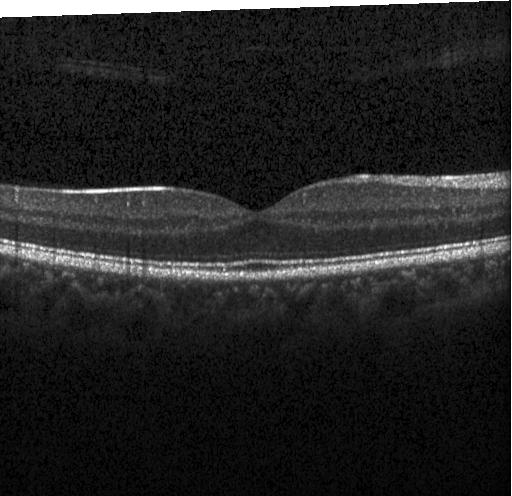 Optical coherence tomography scan — Macular OCT: no choroidal neovascularization, no diabetic macular edema, and no drusen.